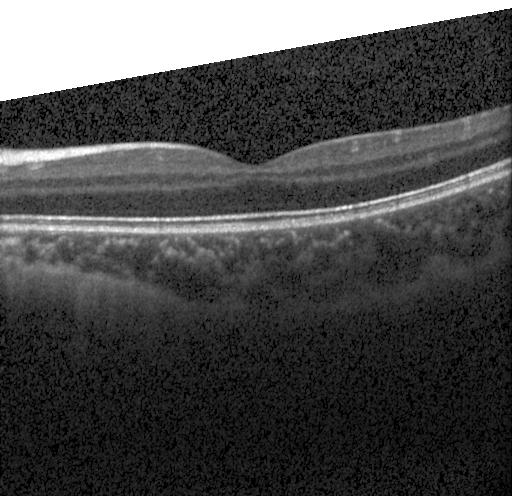

Through the macula · retinal OCT cross-section · SD-OCT — Assessment: neither CNV, DME, nor drusen.